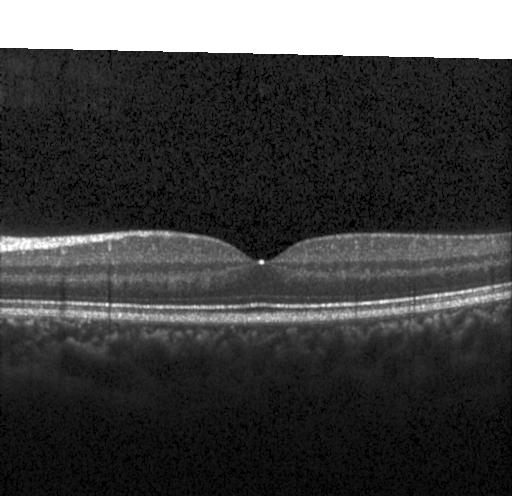
Heidelberg Spectralis · spectral-domain OCT · optical coherence tomography B-scan
Diagnosis: no choroidal neovascularization, diabetic macular edema, or drusen.